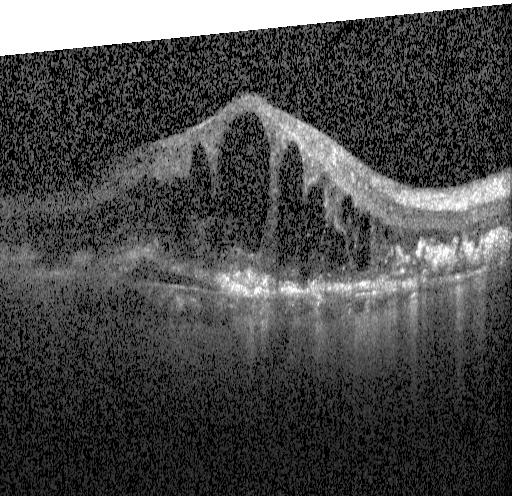
Diagnosis: a choroidal neovascular membrane.